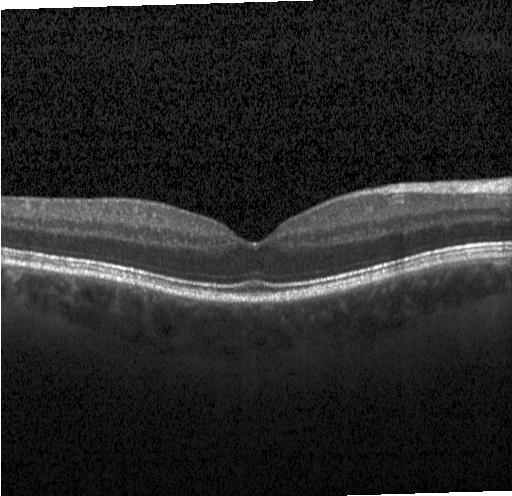 Optical coherence tomography scan
Assessment: no CNV, DME, or drusen.